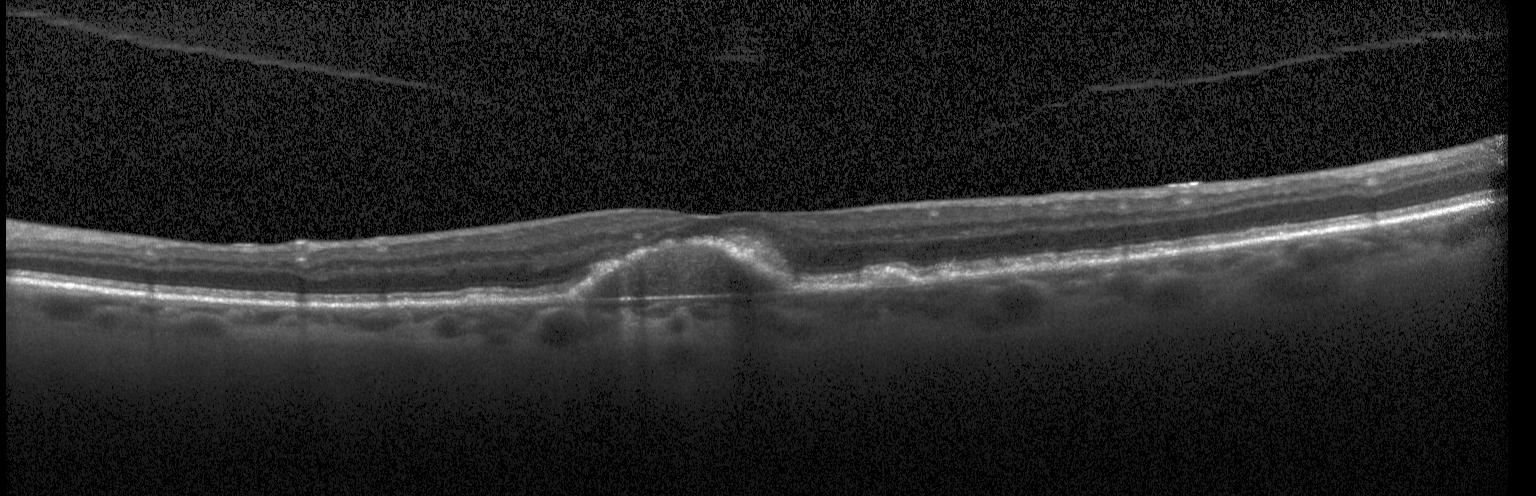

Fovea-centered. SD-OCT. Optical coherence tomography B-scan. Acquired on a Heidelberg Spectralis — Macular OCT: a choroidal neovascular membrane.